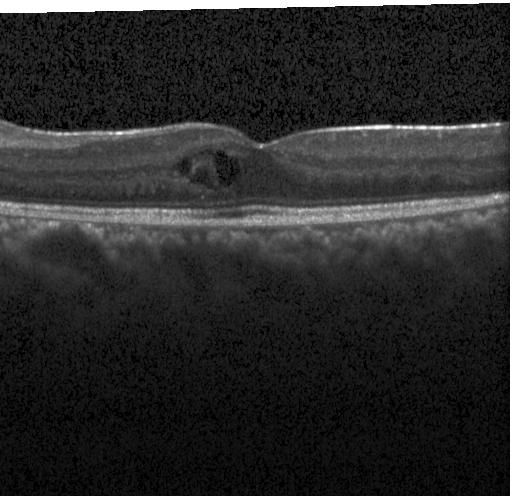

Centered on the fovea; spectral-domain OCT; retinal OCT cross-section. This B-scan demonstrates DME.